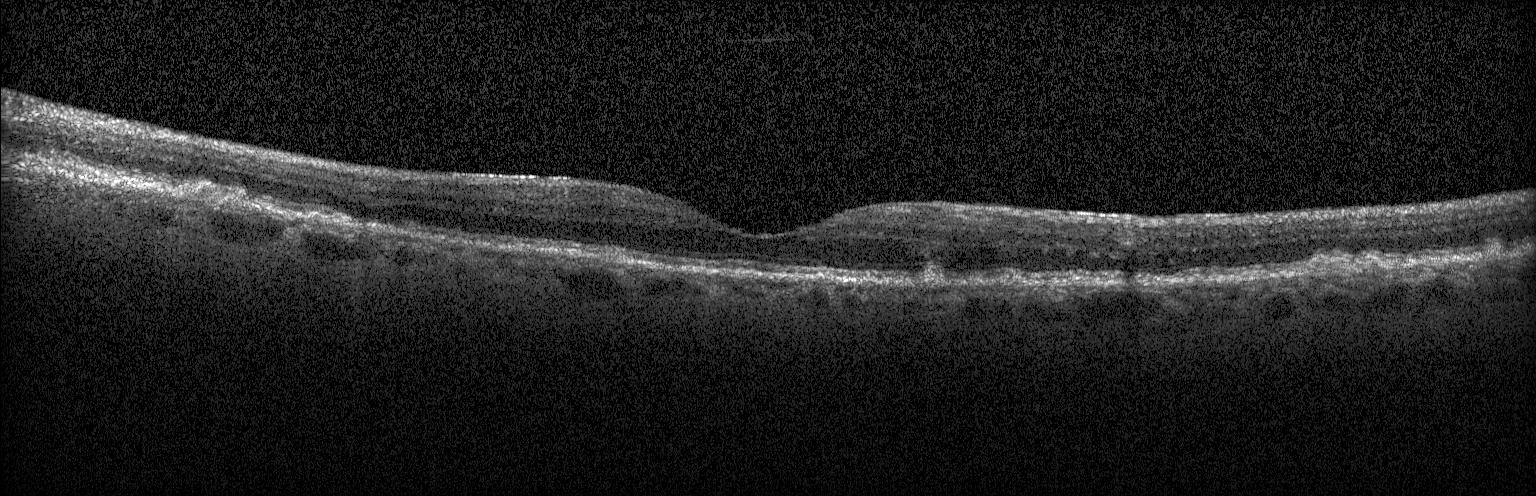

OCT line scan, Heidelberg Spectralis.
Impression: drusen.